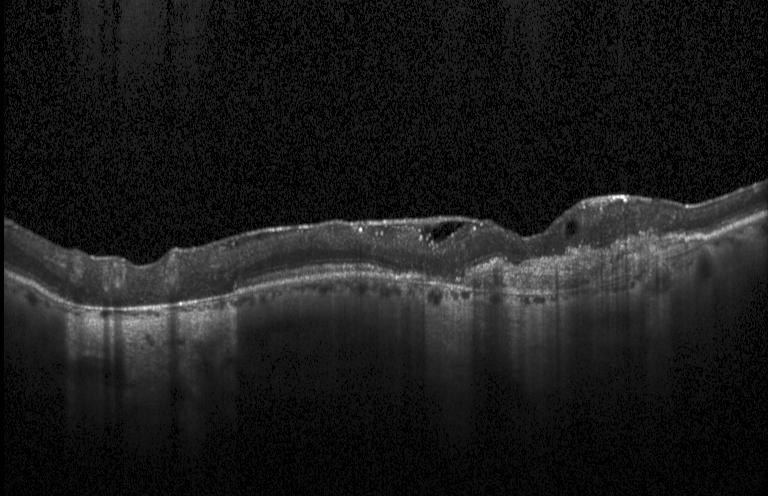 Optical coherence tomography B-scan. Dx: choroidal neovascularization.